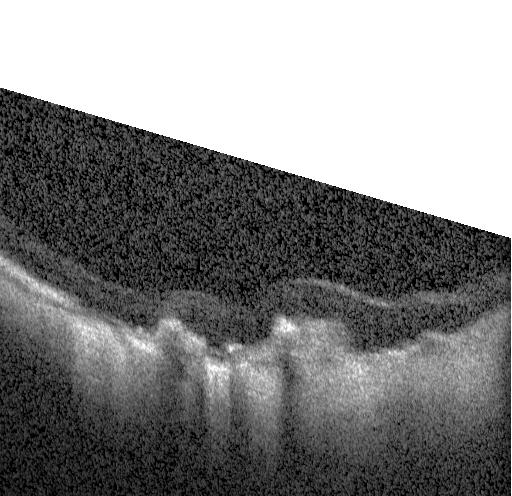 Impression: choroidal neovascularization.